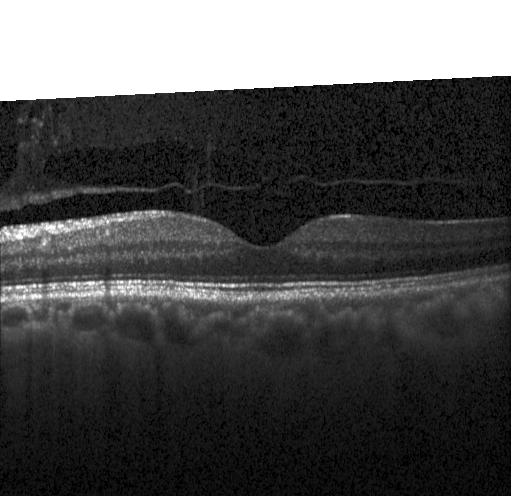

No evidence of choroidal neovascularization, diabetic macular edema, or drusen.